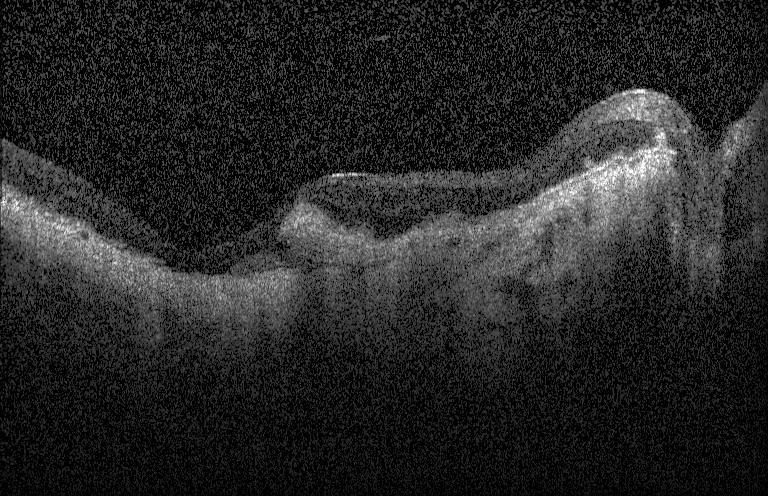 Macular OCT: choroidal neovascularization (CNV).